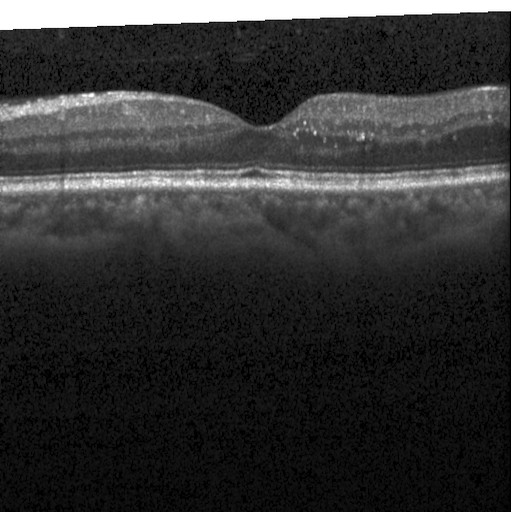

Retinal OCT cross-section — This B-scan demonstrates diabetic macular edema.